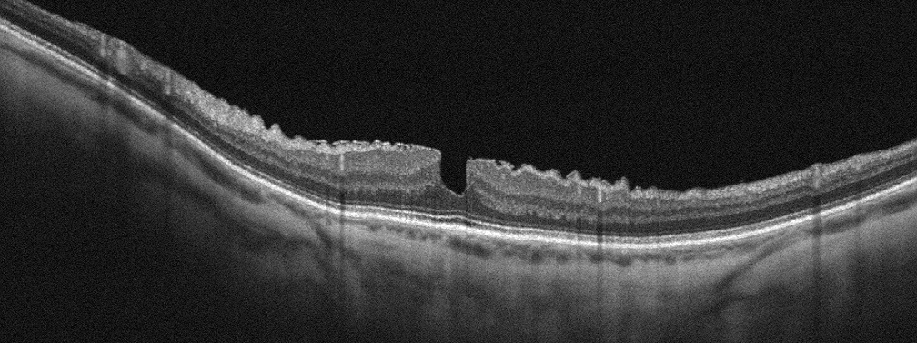 Retinal OCT B-scan. Instrument: Optovue Avanti RTVue XR. Diagnosis: ERM.